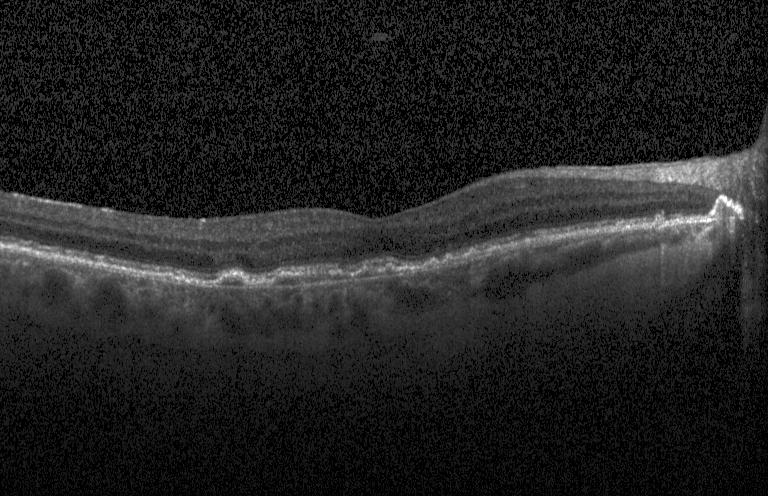 Macular OCT: CNV.